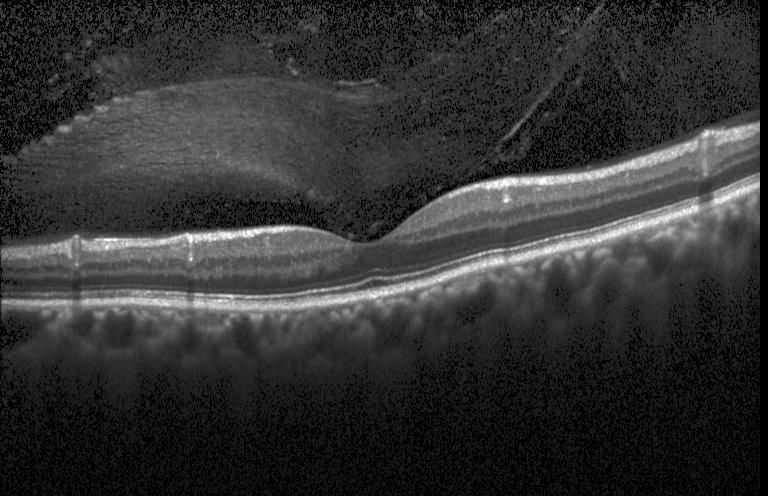 OCT line scan · spectral-domain OCT
OCT finding: no evidence of CNV, DME, or drusen.